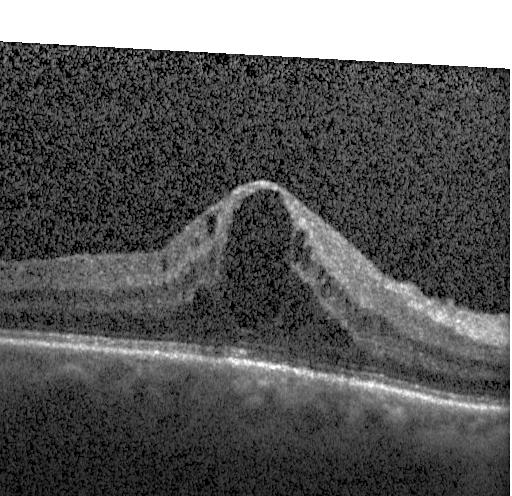 Optical coherence tomography B-scan; spectral-domain OCT. Diagnosis: diabetic macular edema.